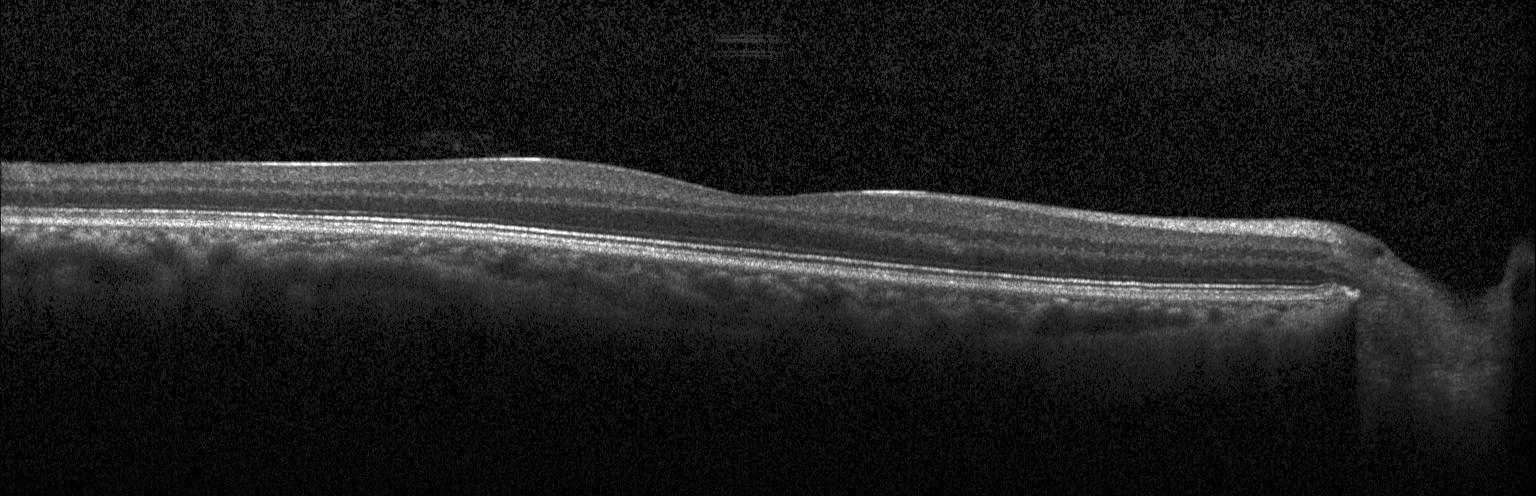 OCT B-scan showing no CNV, DME, or drusen.